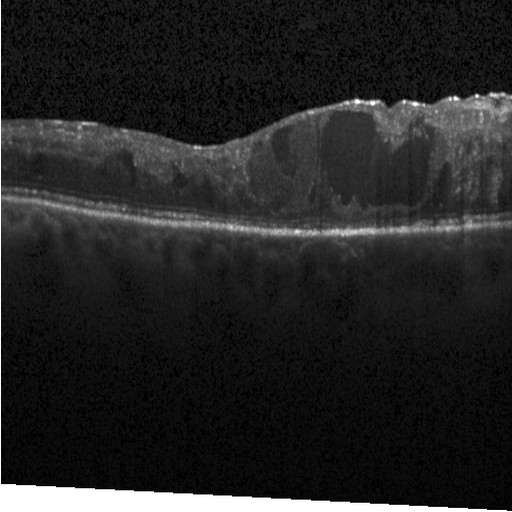
Dx: diabetic macular edema.